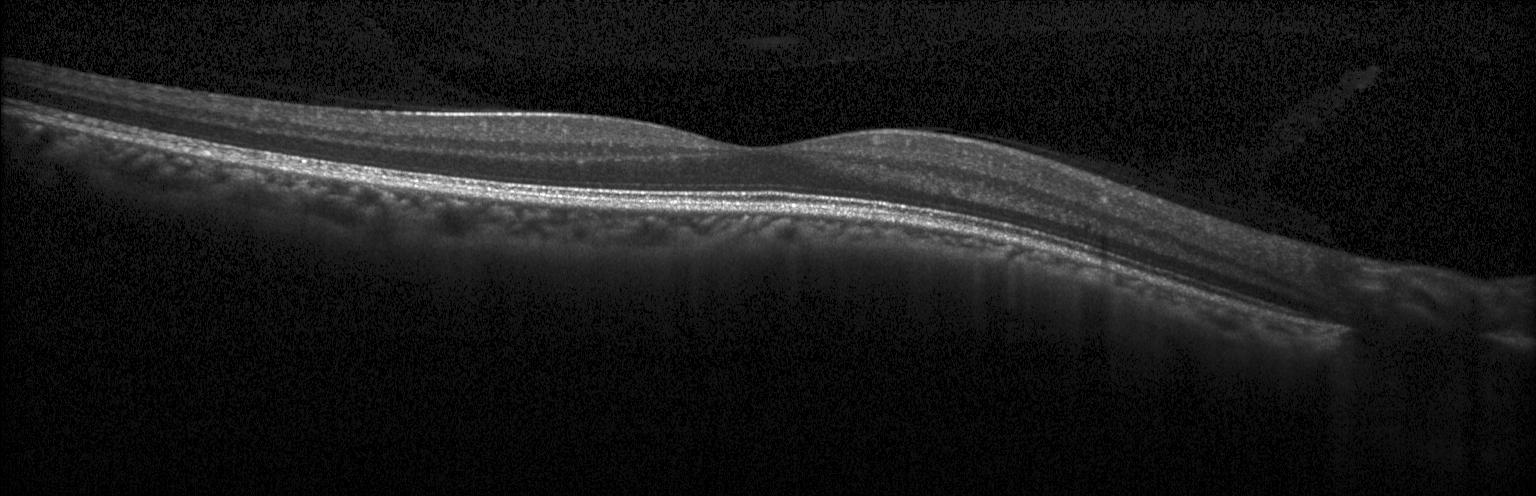
OCT line scan.
Assessment: no choroidal neovascularization, diabetic macular edema, or drusen.